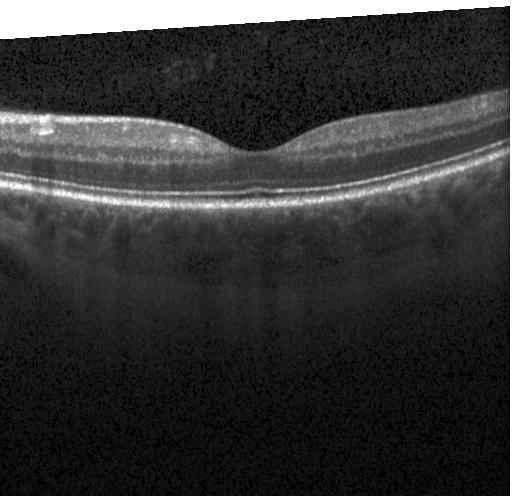
OCT B-scan · Heidelberg Spectralis. OCT finding: neither choroidal neovascularization, diabetic macular edema, nor drusen.